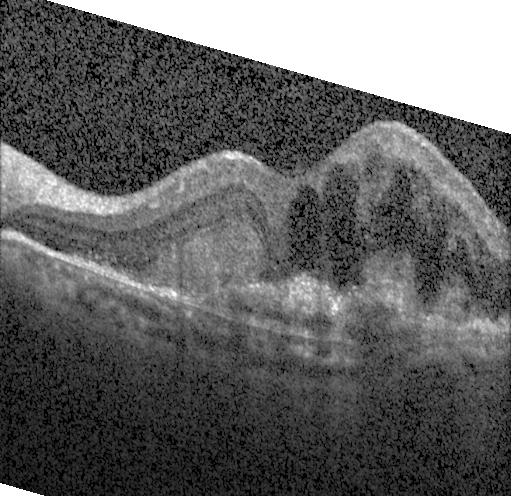

Diagnosis: choroidal neovascularization.